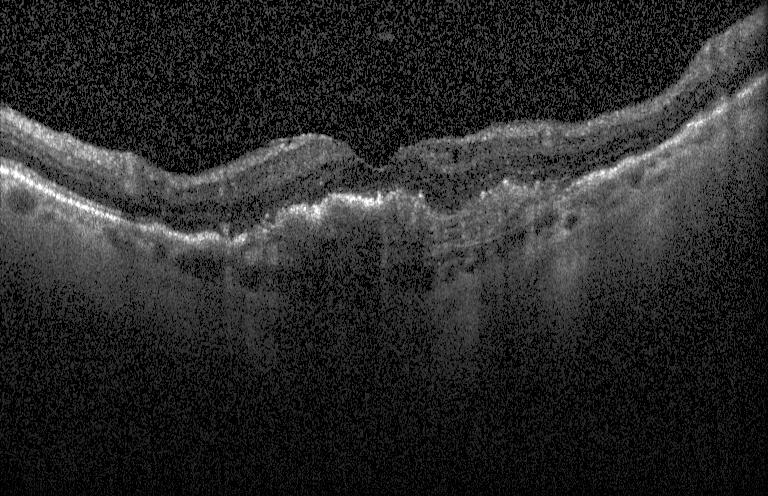

OCT line scan.
This B-scan demonstrates a choroidal neovascular membrane.